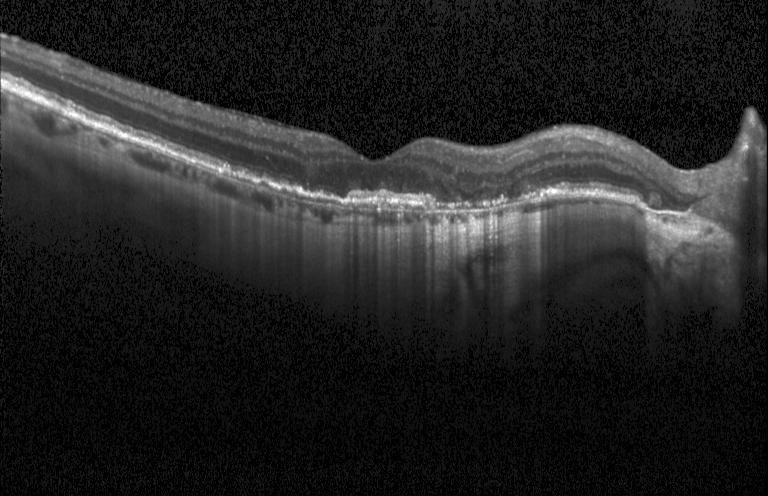
Heidelberg Spectralis OCT system, optical coherence tomography scan, spectral-domain optical coherence tomography — This B-scan demonstrates a choroidal neovascular membrane.